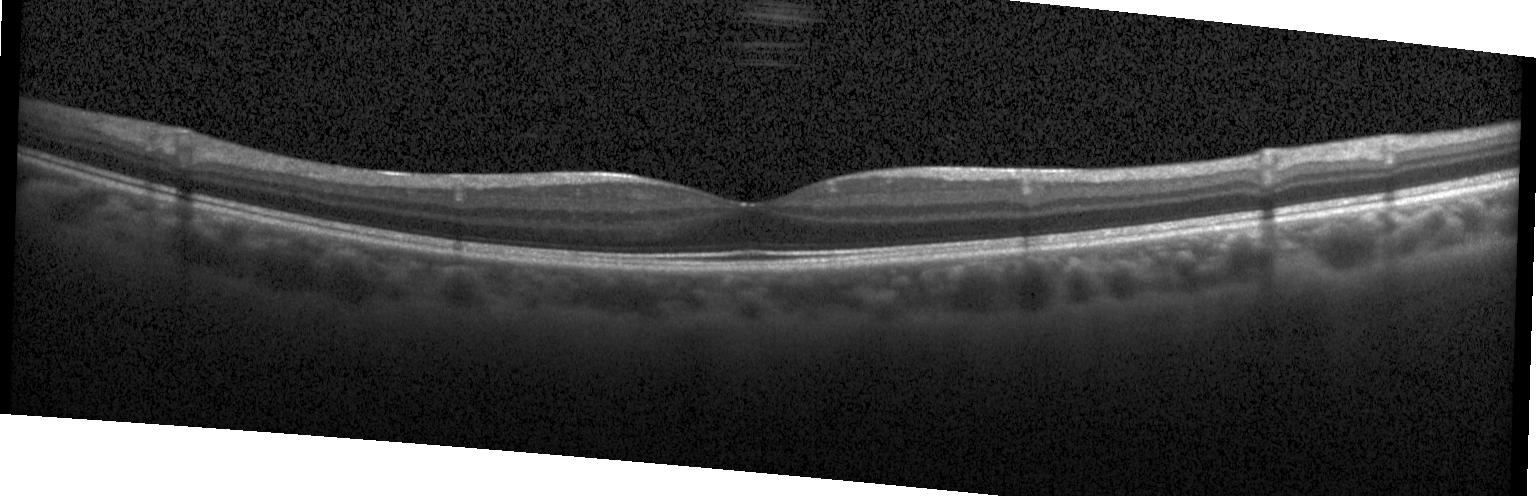
Retinal OCT cross-section, Heidelberg Spectralis.
Diagnosis: no evidence of choroidal neovascularization, diabetic macular edema, or drusen.